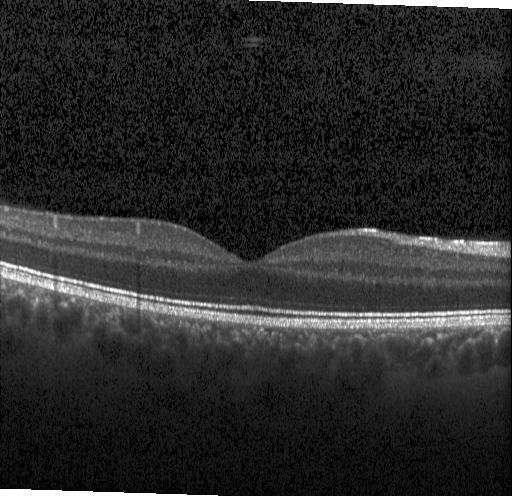

Horizontal scan through the fovea; retinal OCT cross-section. The scan shows no CNV, DME, or drusen.